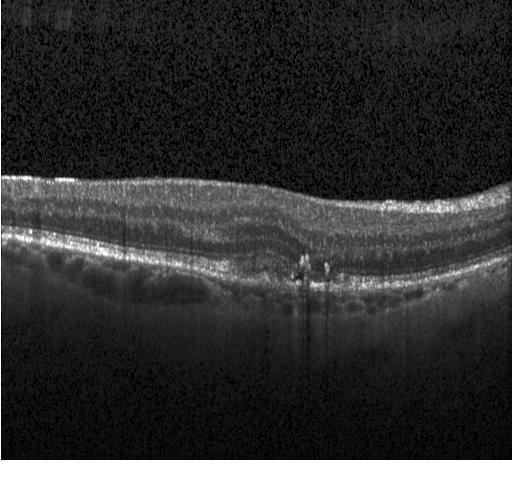

OCT line scan.
OCT finding: a choroidal neovascular membrane.